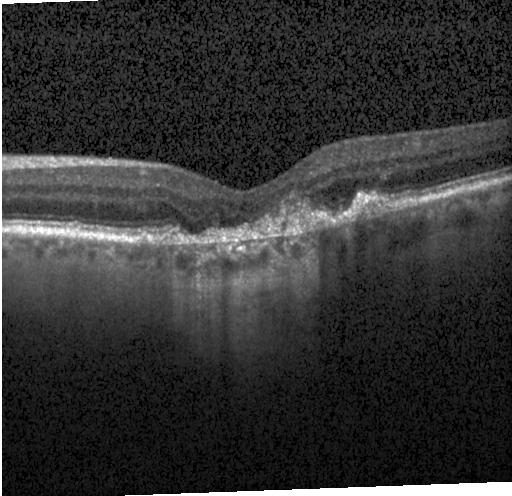

OCT line scan.
Diagnosis: choroidal neovascularization.